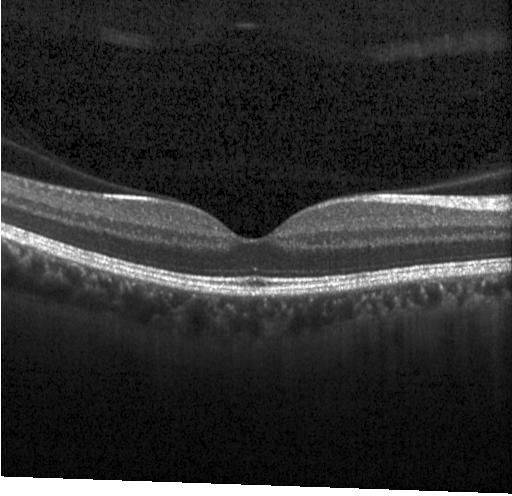 Spectral-domain OCT. Retinal OCT B-scan — Finding: no choroidal neovascularization, no diabetic macular edema, and no drusen.